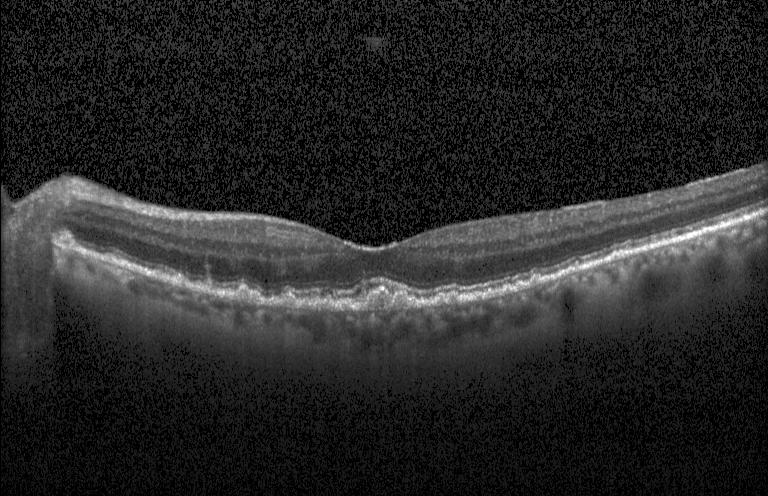

Through the macula · OCT B-scan · spectral-domain OCT · Heidelberg Spectralis OCT system.
Impression: drusen.